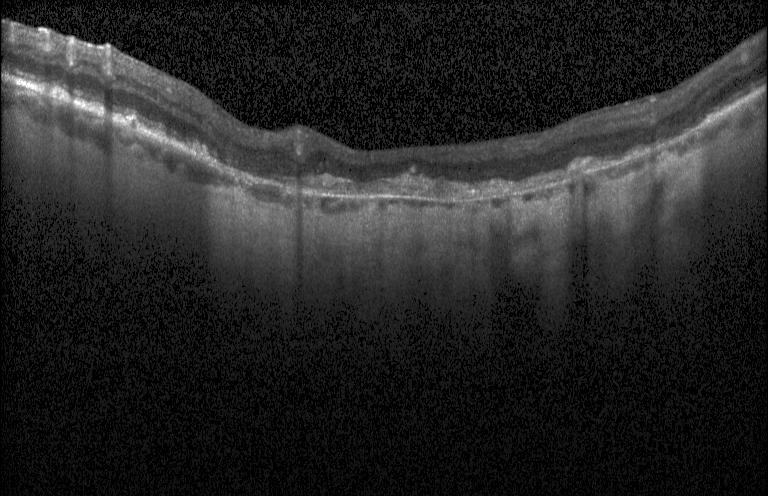
OCT line scan. Through the macula. Finding: choroidal neovascularization (CNV).